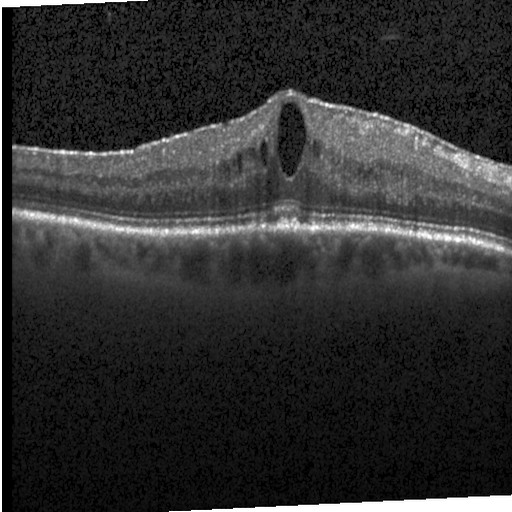
OCT line scan. Heidelberg Spectralis OCT system. Spectral-domain OCT
Finding: diabetic macular edema (DME).